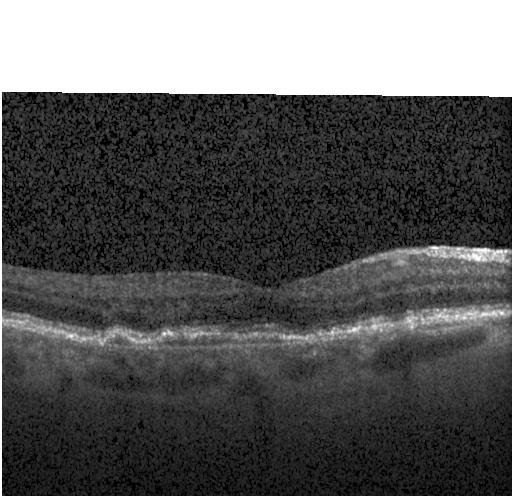
Finding: a choroidal neovascular membrane.